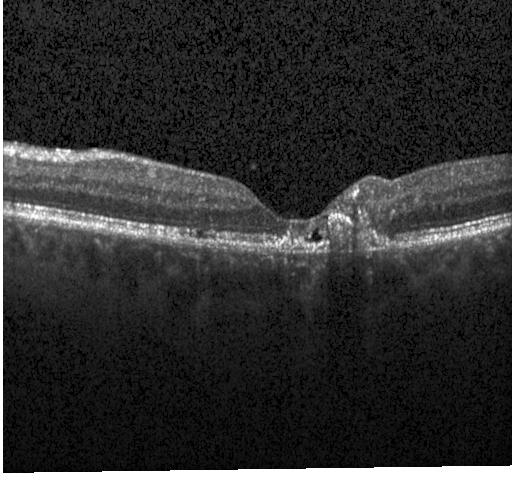
Retinal OCT cross-section, Heidelberg Spectralis OCT system, centered on the fovea.
Macular OCT: a choroidal neovascular membrane.